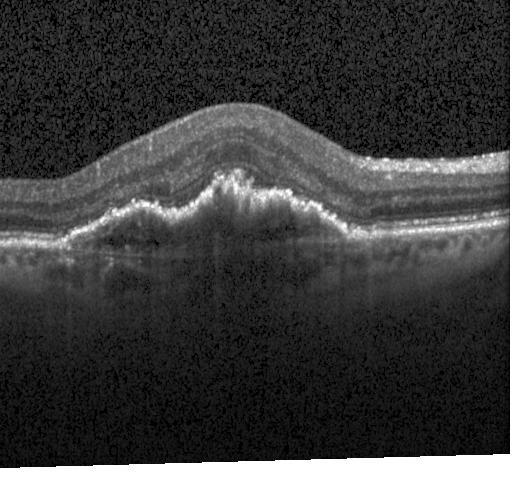

OCT B-scan. Heidelberg Spectralis. Through the macula. Spectral-domain optical coherence tomography — Diagnosis: a choroidal neovascular membrane.